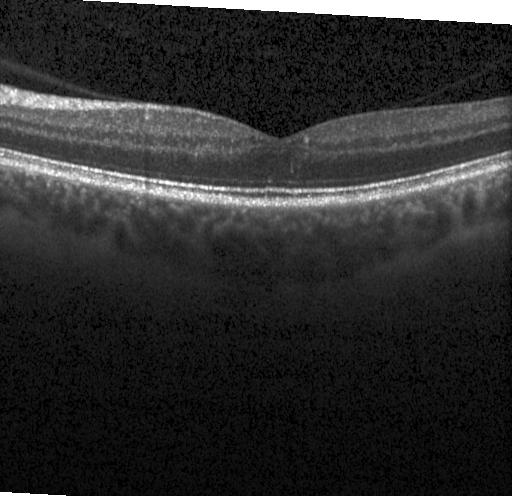

Retinal OCT cross-section.
Macular OCT: no choroidal neovascularization, no diabetic macular edema, and no drusen.